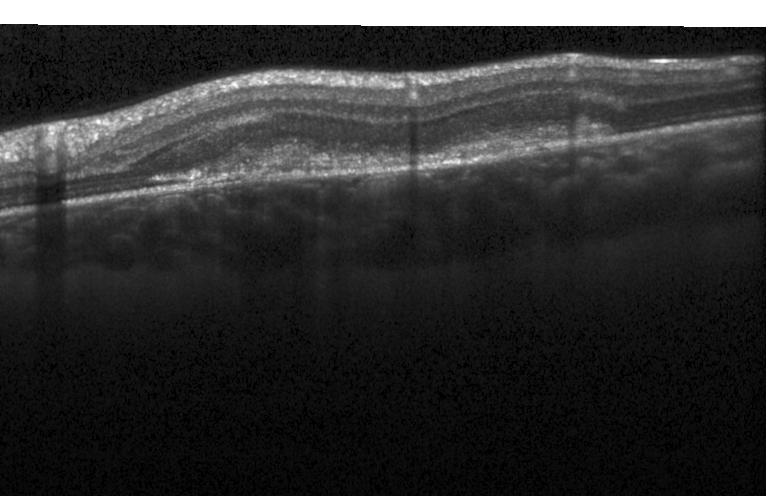

OCT finding: a choroidal neovascular membrane.